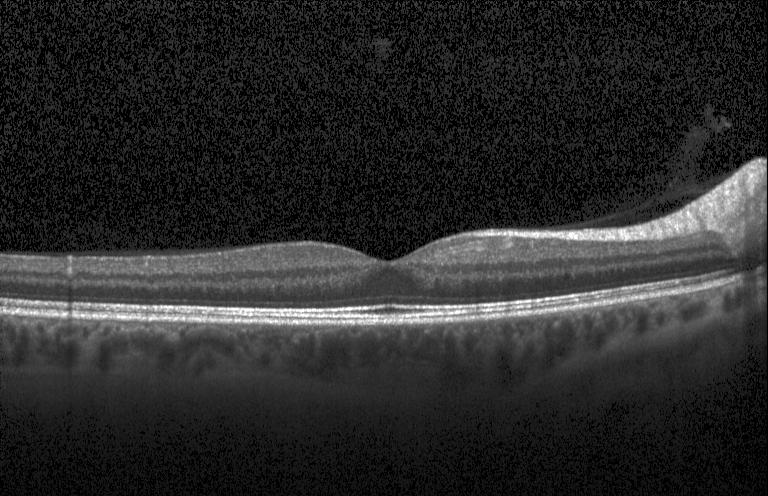
Finding: no CNV, DME, or drusen.